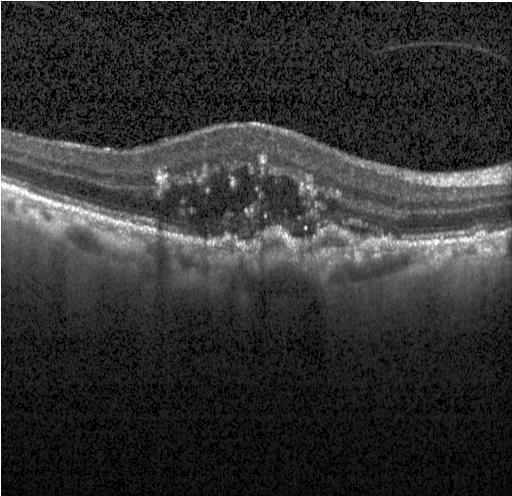
Retinal OCT cross-section. Heidelberg Spectralis OCT system. Spectral-domain optical coherence tomography. Through the macula
Finding: choroidal neovascularization.